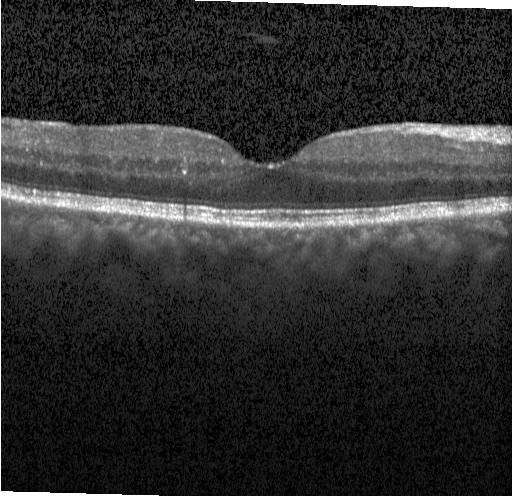 OCT B-scan showing no evidence of CNV, DME, or drusen.